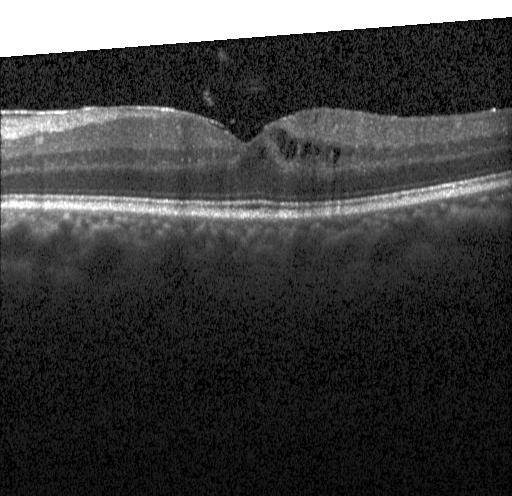
OCT finding: diabetic macular edema (DME).